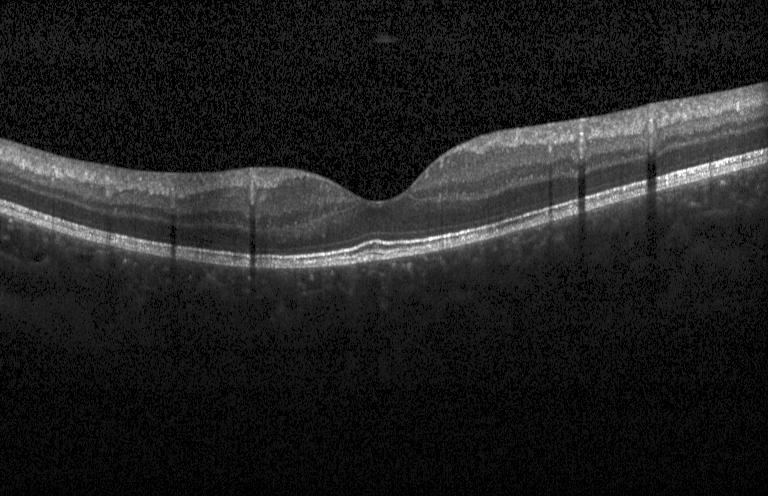 SD-OCT; Heidelberg Spectralis; optical coherence tomography scan.
Finding: neither CNV, DME, nor drusen.